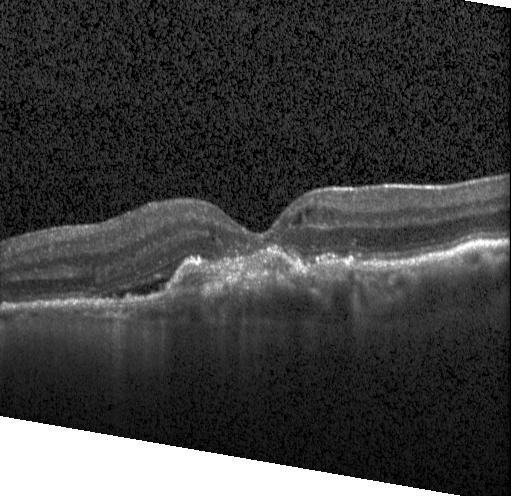
Spectral-domain OCT; optical coherence tomography scan; horizontal scan through the fovea; instrument: Heidelberg Spectralis.
This B-scan demonstrates a choroidal neovascular membrane.